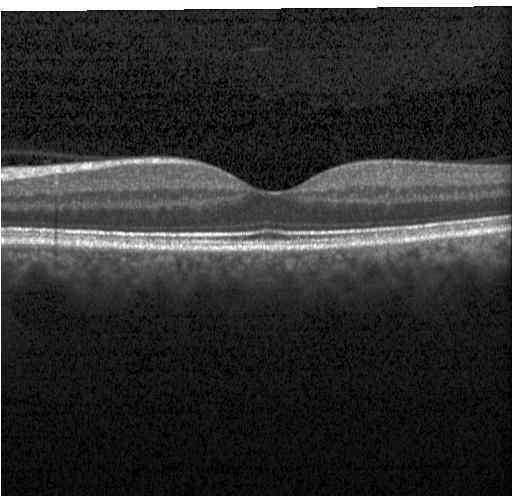

Centered on the fovea, acquired on a Heidelberg Spectralis, OCT B-scan.
Macular OCT: no CNV, no DME, and no drusen.